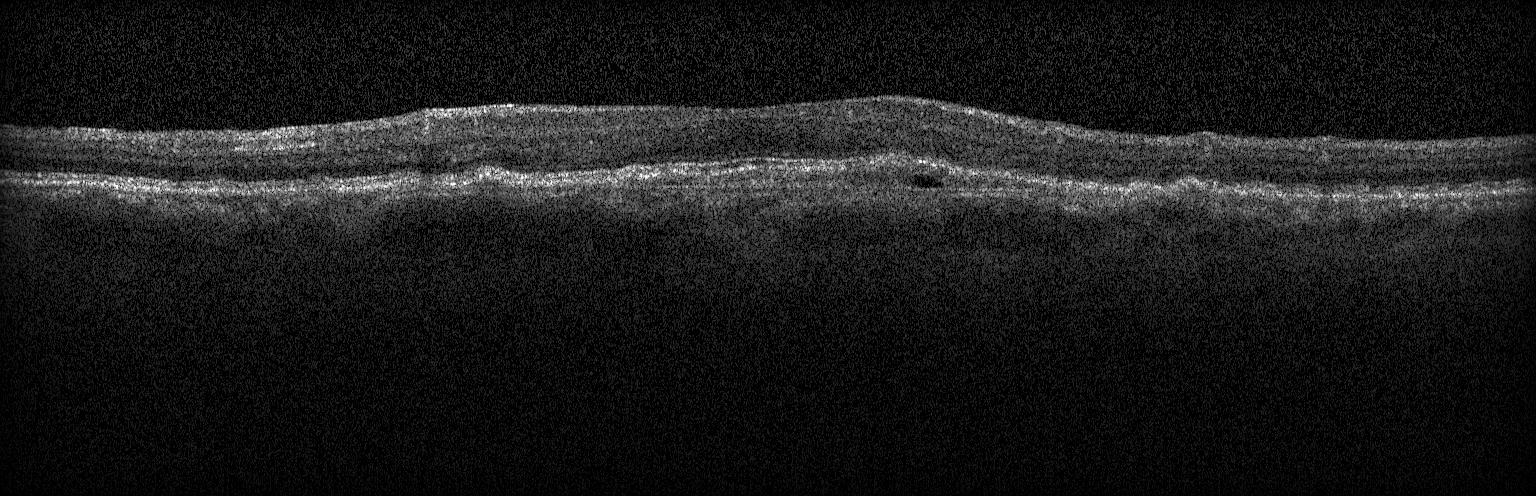 OCT B-scan showing a choroidal neovascular membrane.